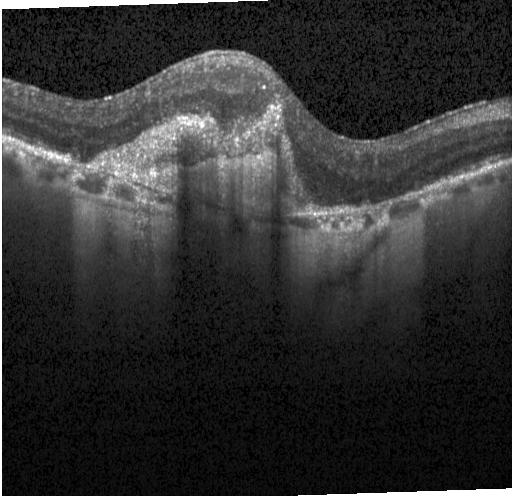 OCT line scan, acquired on a Heidelberg Spectralis, through the macula. Macular OCT: a choroidal neovascular membrane.